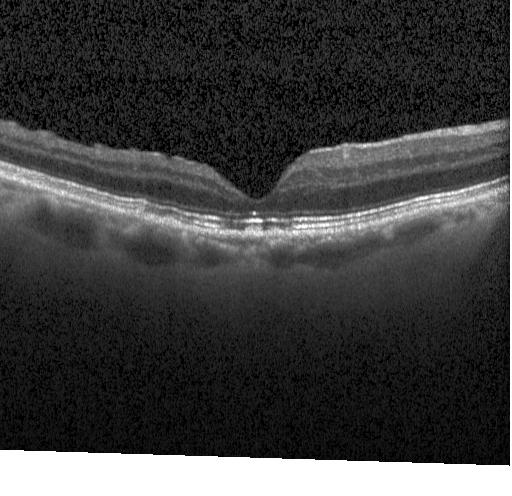

Finding: no choroidal neovascularization, diabetic macular edema, or drusen.